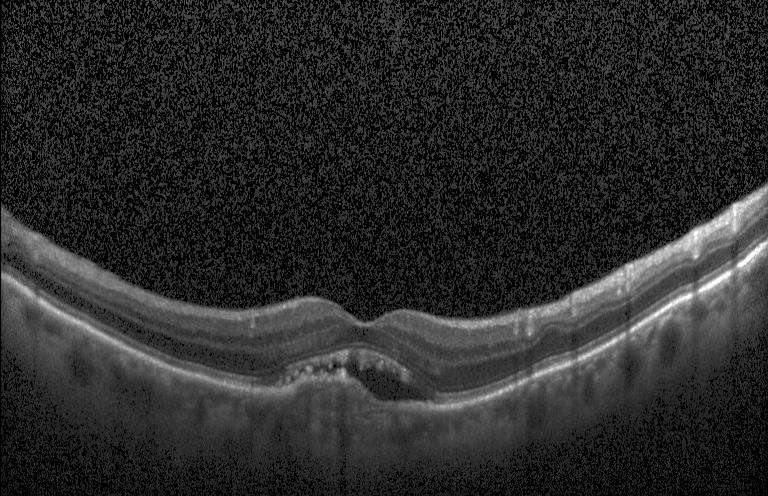
SD-OCT, retinal OCT cross-section — Choroidal neovascularization (CNV).